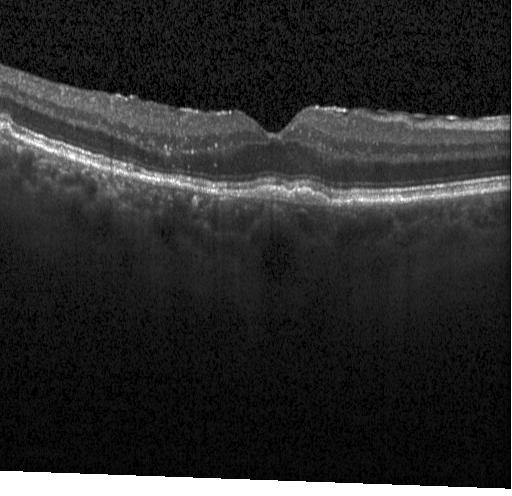 OCT scan showing choroidal neovascularization.